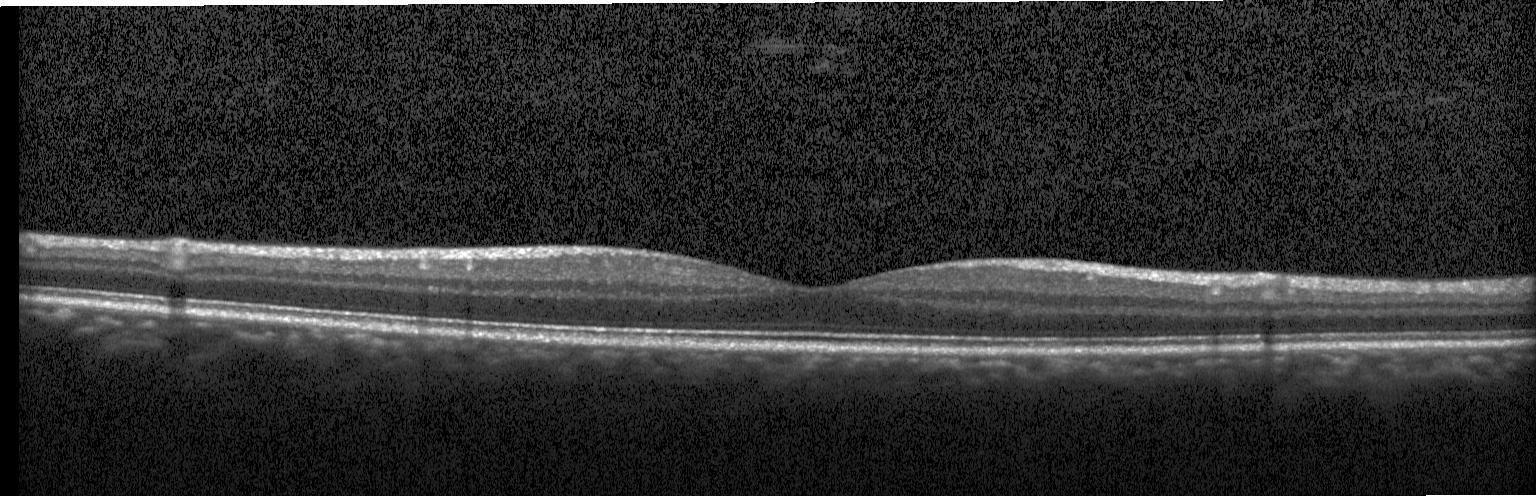

SD-OCT; optical coherence tomography B-scan; fovea-centered.
Impression: neither choroidal neovascularization, diabetic macular edema, nor drusen.